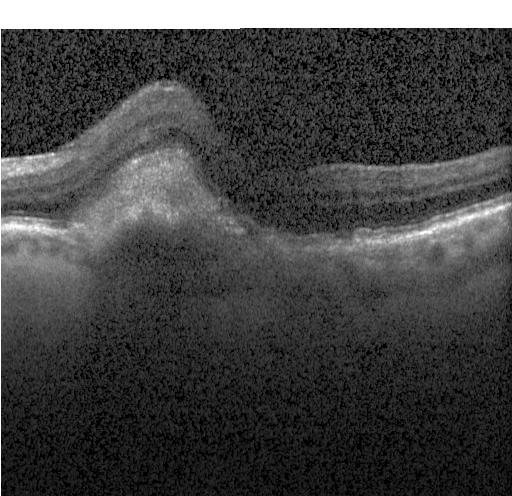 Fovea-centered; optical coherence tomography scan
Diagnosis: CNV.